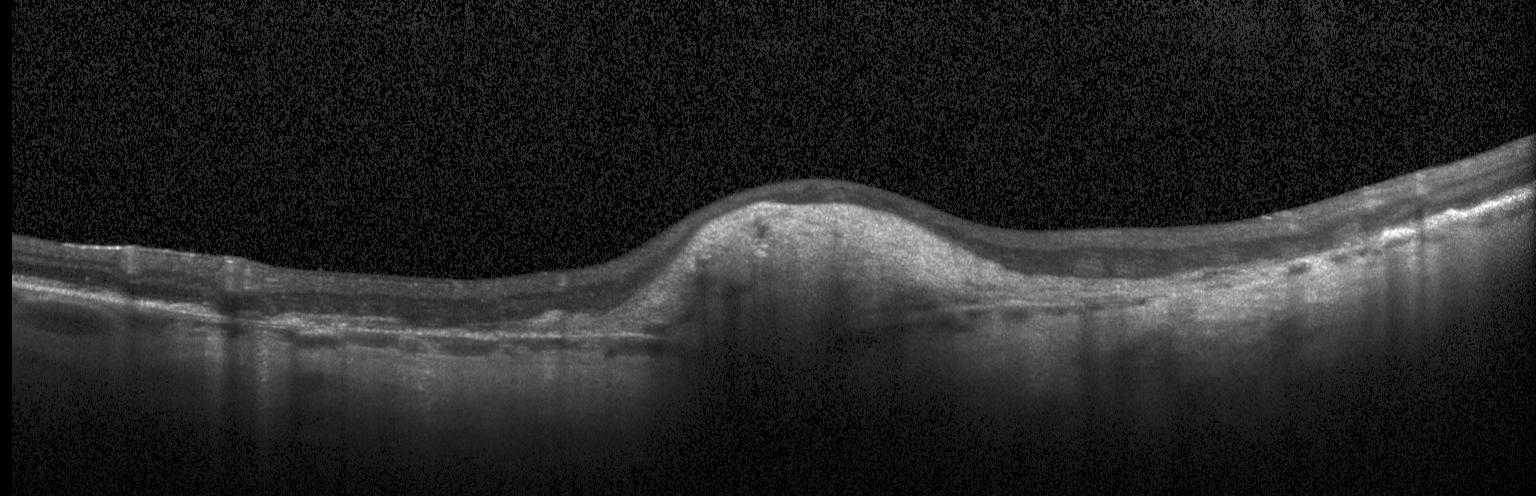 Heidelberg Spectralis OCT system · spectral-domain OCT · centered on the fovea · retinal OCT B-scan.
CNV.